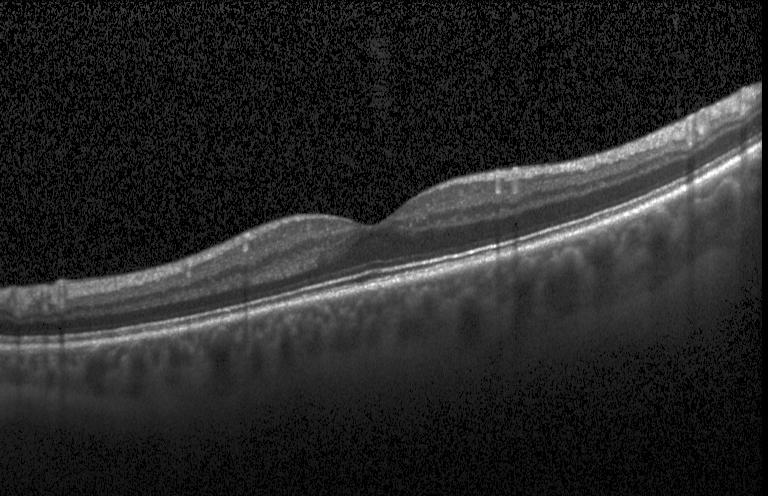

The scan shows no CNV, no DME, and no drusen.